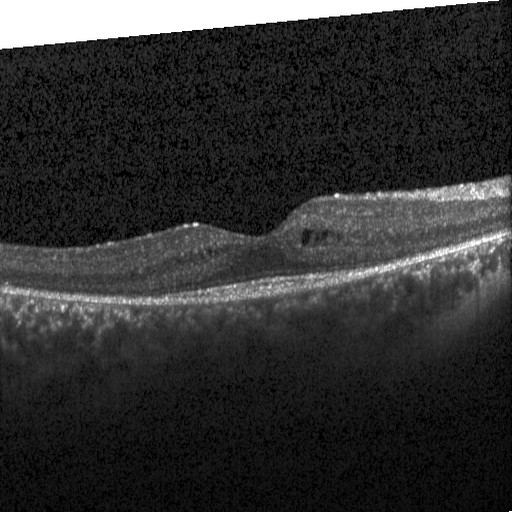

OCT B-scan · SD-OCT · fovea-centered · Heidelberg Spectralis OCT system — Assessment: diabetic macular edema.